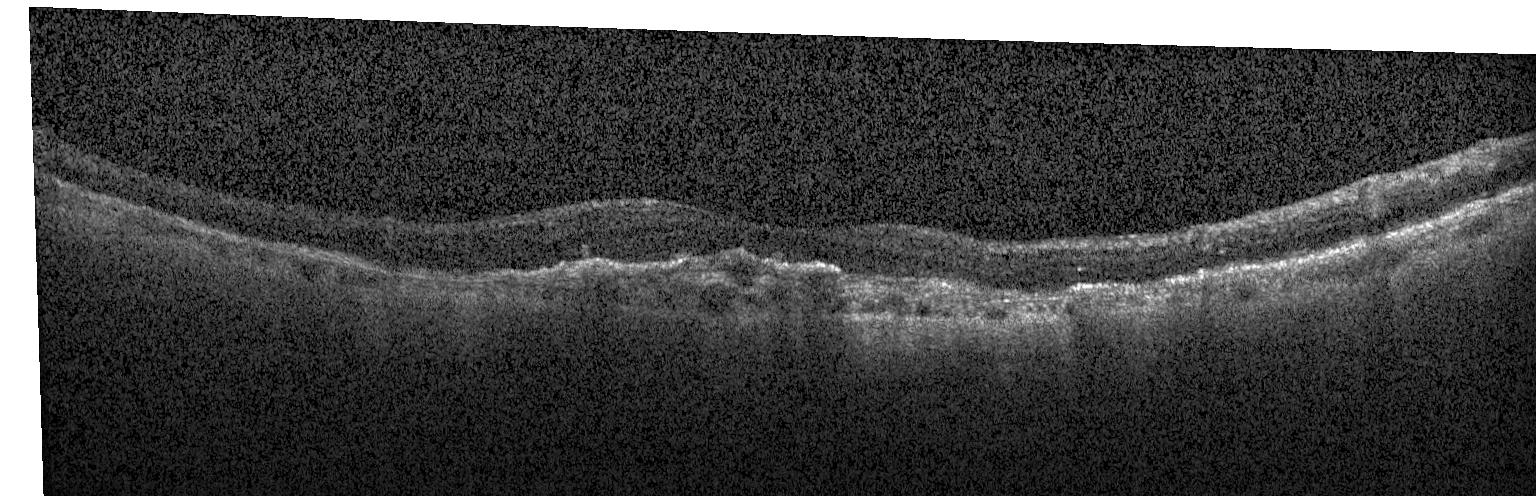
OCT scan showing a choroidal neovascular membrane.